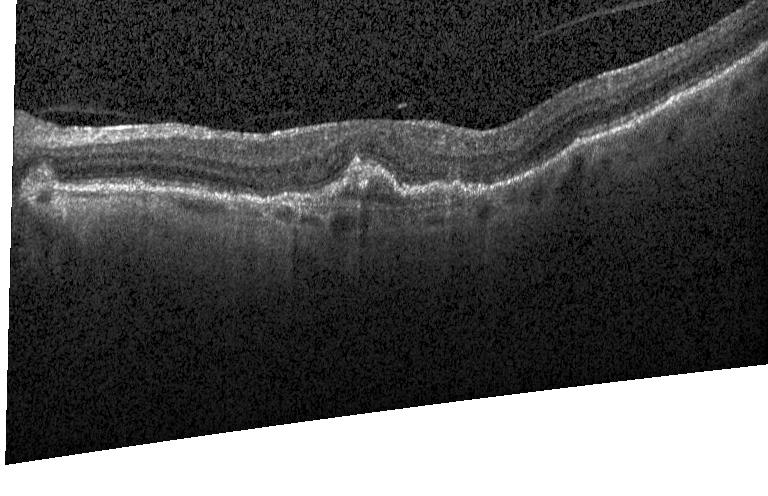

OCT B-scan showing a choroidal neovascular membrane.